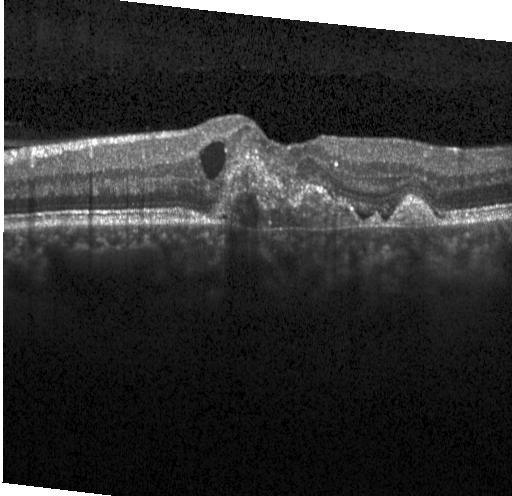 Retinal OCT B-scan. The scan shows a choroidal neovascular membrane.